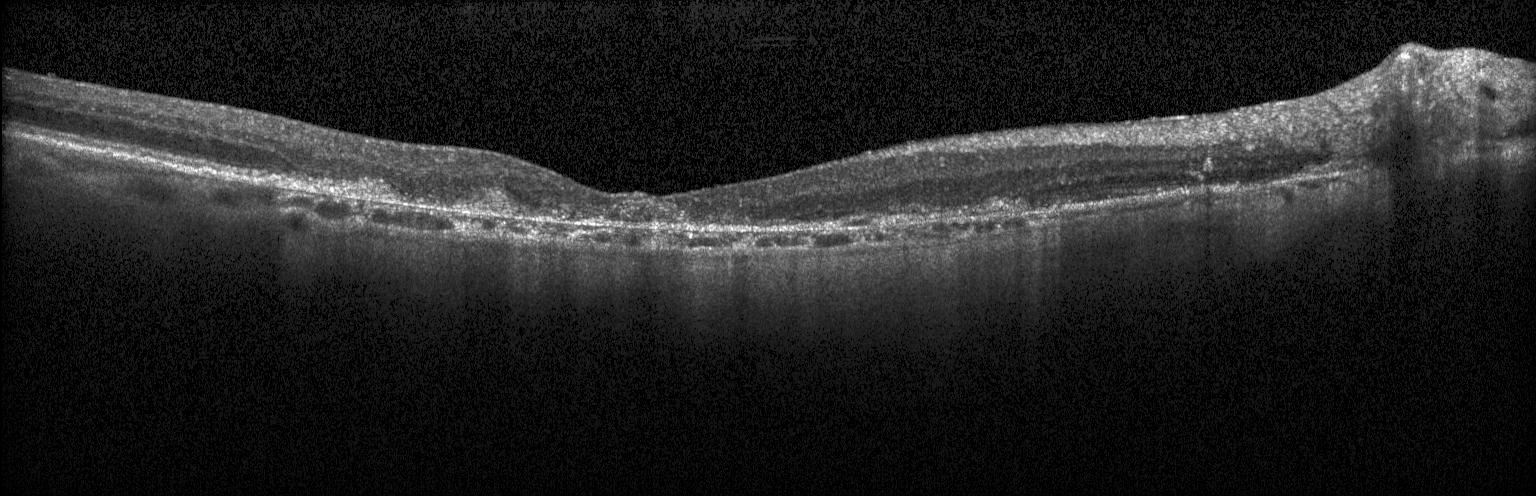 Optical coherence tomography B-scan. Finding: a choroidal neovascular membrane.